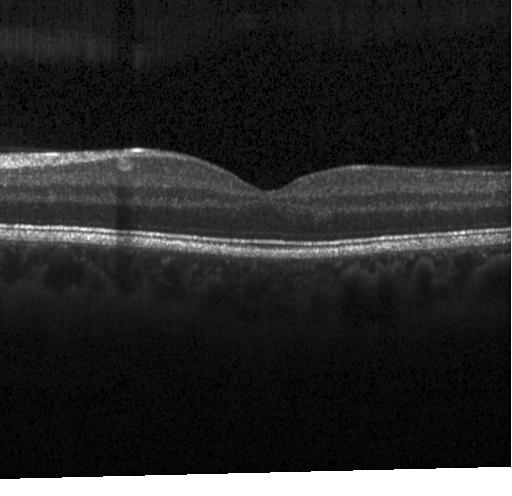 Horizontal scan through the fovea · optical coherence tomography B-scan
The scan shows no choroidal neovascularization, no diabetic macular edema, and no drusen.